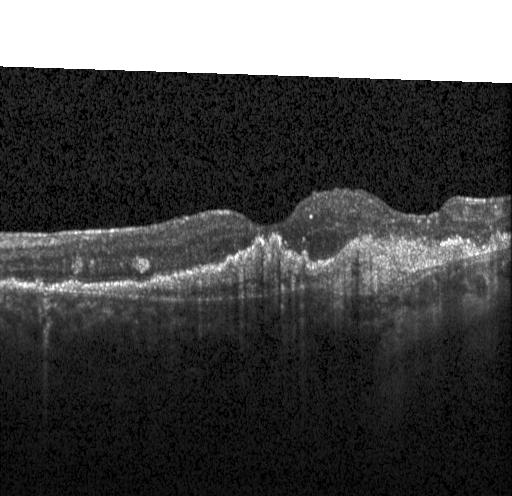

OCT line scan. Choroidal neovascularization (CNV).